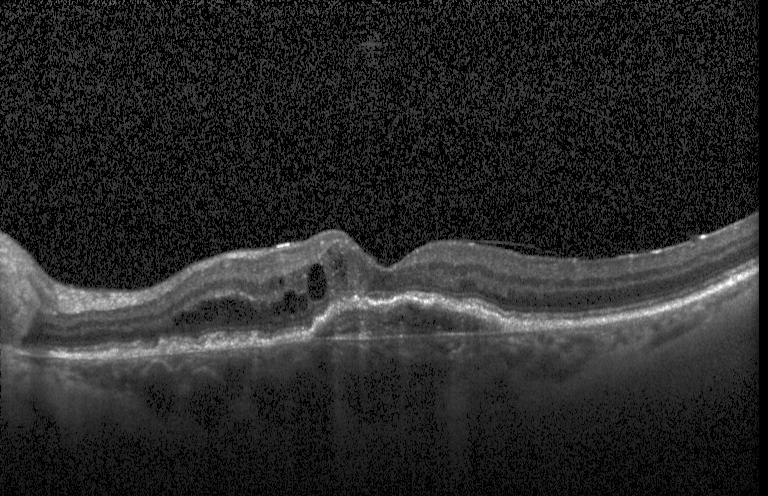 Spectral-domain optical coherence tomography. Heidelberg Spectralis. Optical coherence tomography scan.
Diagnosis: choroidal neovascularization.